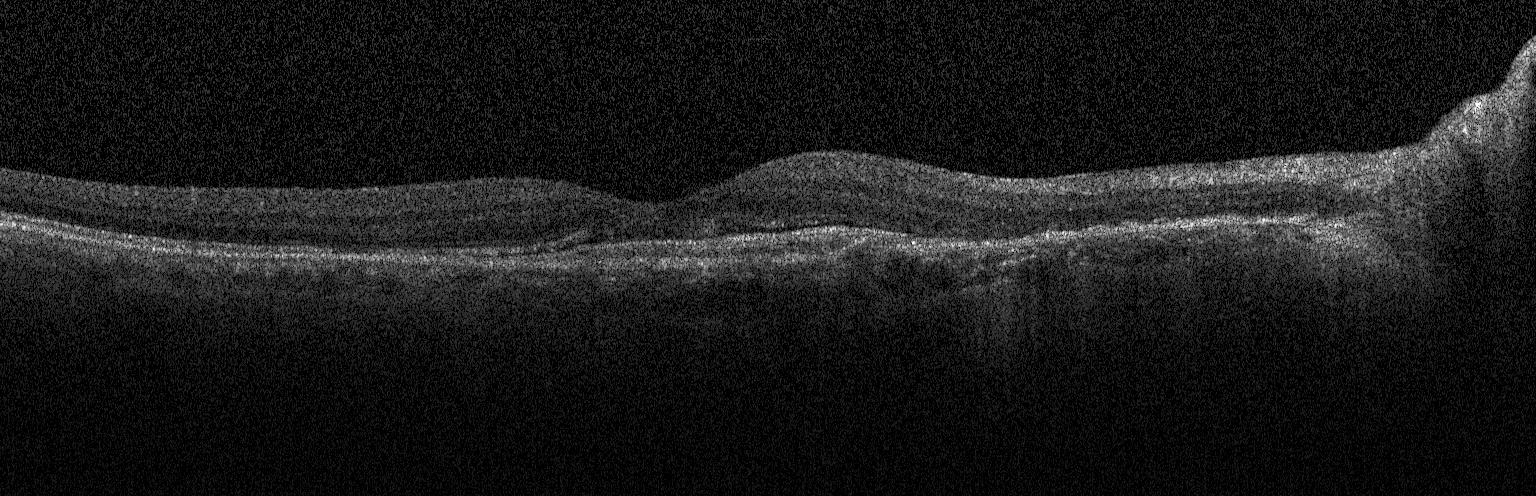

SD-OCT, OCT B-scan
The scan shows choroidal neovascularization (CNV).